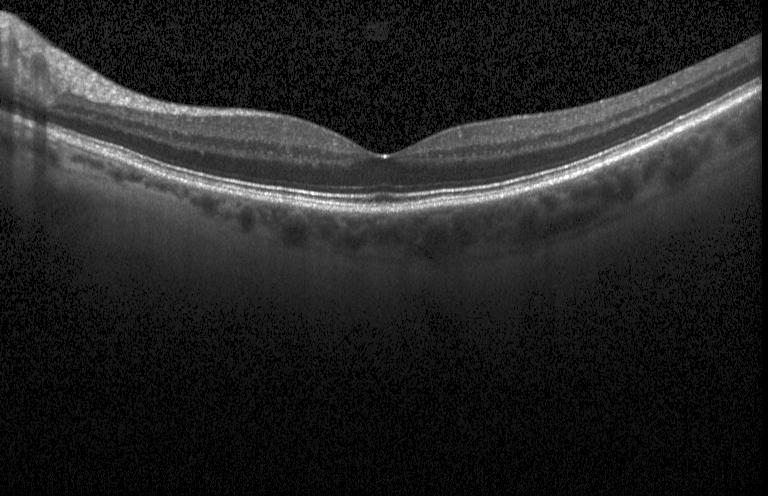
Acquired on a Heidelberg Spectralis. SD-OCT. Optical coherence tomography B-scan — Diagnosis: no evidence of CNV, DME, or drusen.